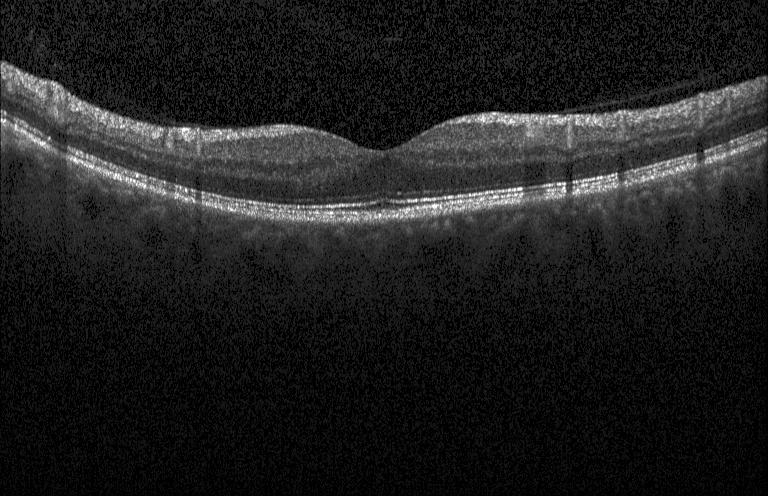 Optical coherence tomography scan.
Finding: no CNV, no DME, and no drusen.